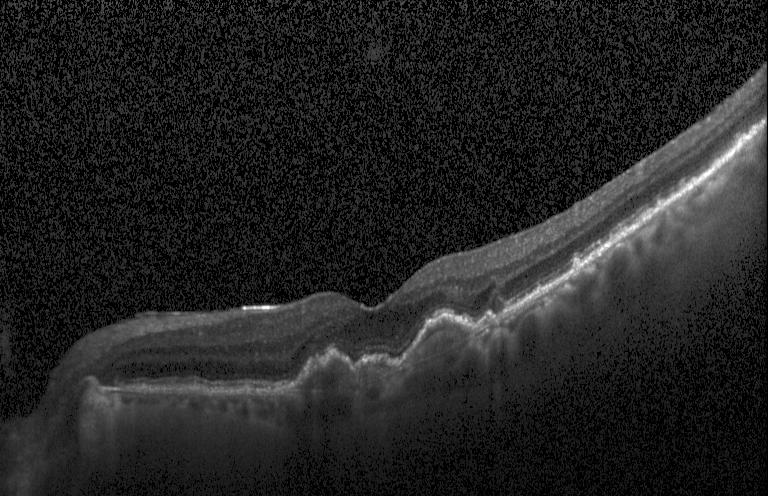
Retinal OCT cross-section showing a choroidal neovascular membrane.